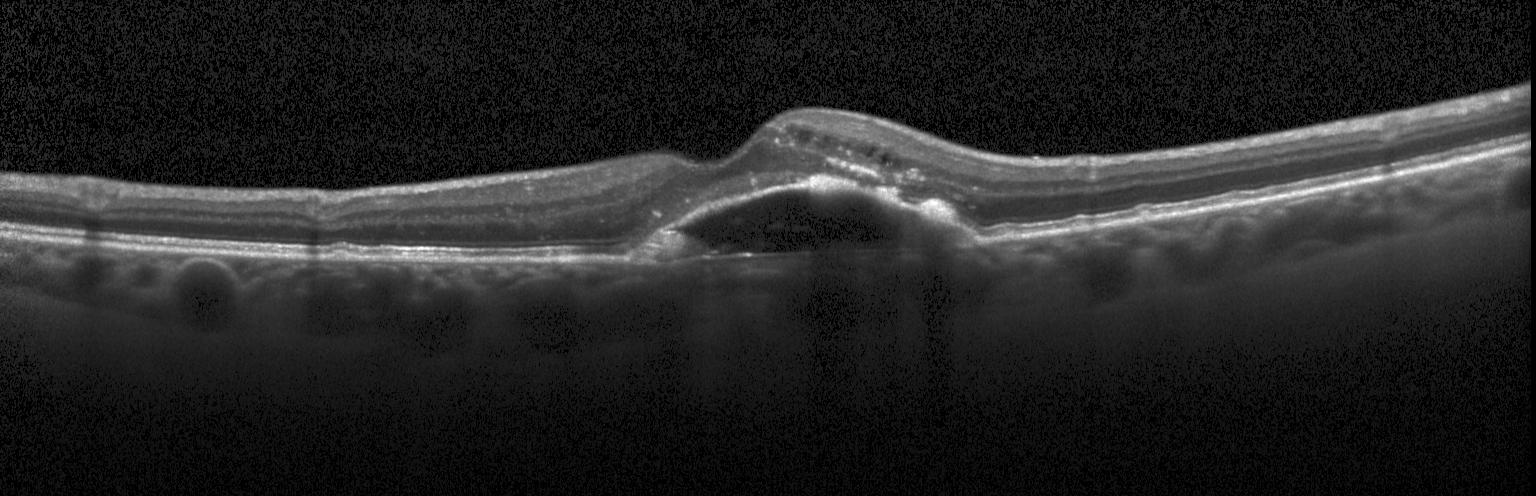 A choroidal neovascular membrane.